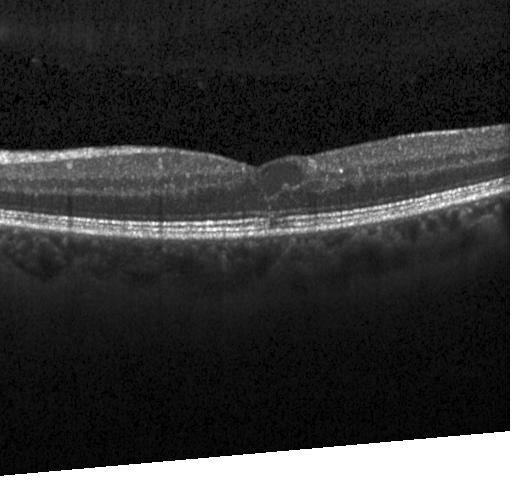

Dx: diabetic macular edema.